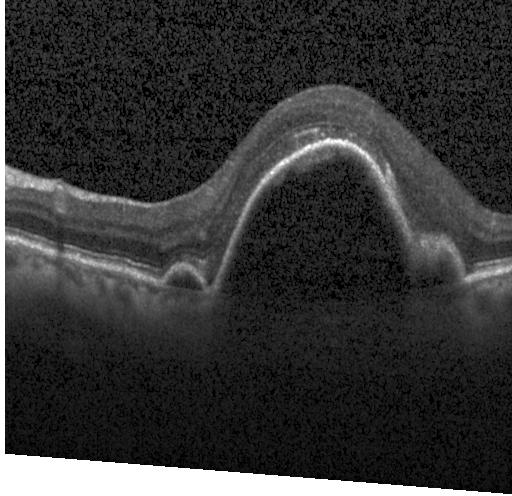
Diagnosis: choroidal neovascularization.